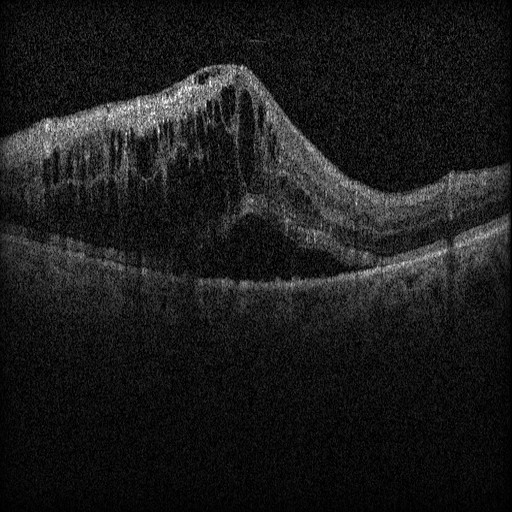

Through the macula. Instrument: Heidelberg Spectralis. Retinal OCT B-scan. Spectral-domain OCT. Assessment: diabetic macular edema.